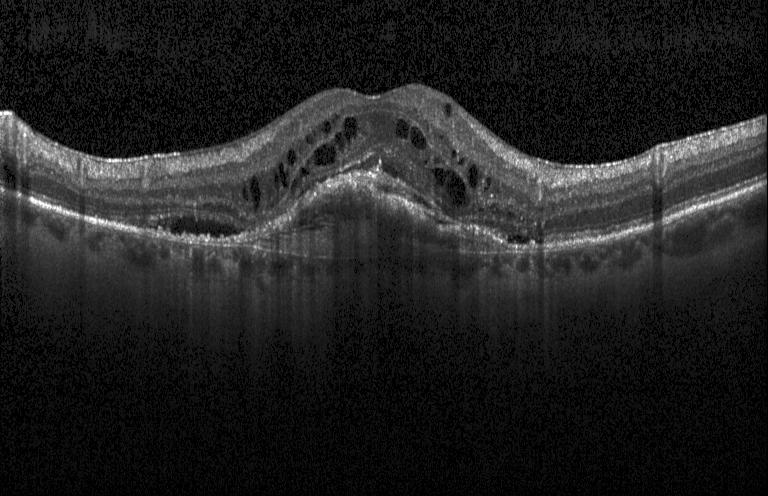

OCT B-scan; spectral-domain OCT. Impression: choroidal neovascularization.